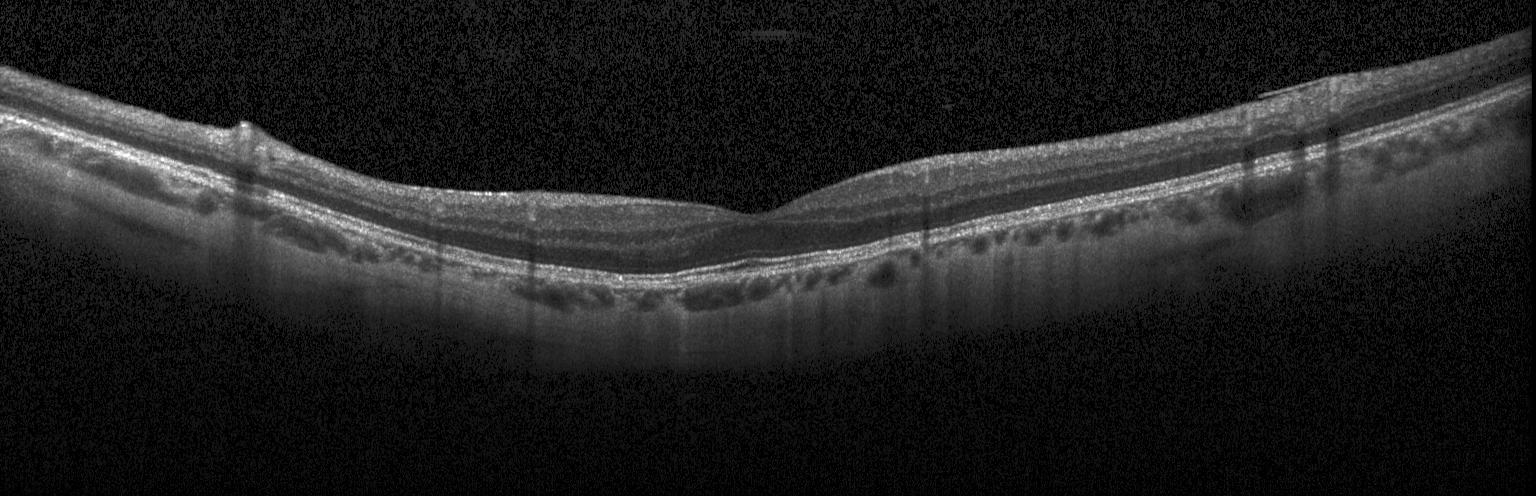 Diagnosis: no choroidal neovascularization, diabetic macular edema, or drusen.